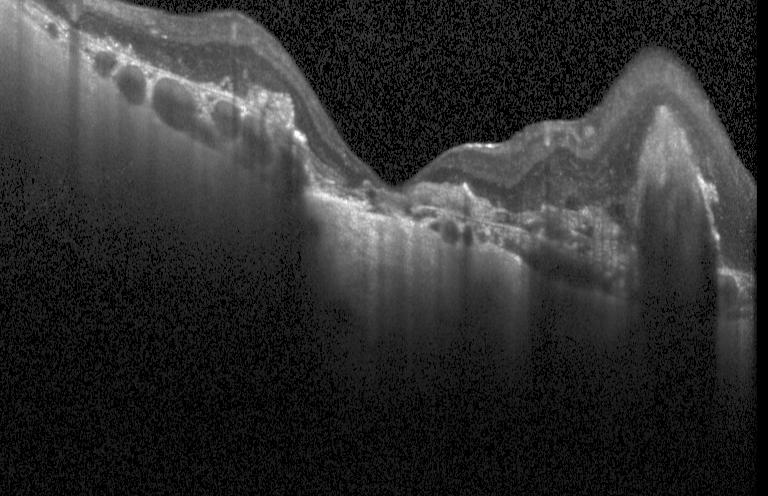
Instrument: Heidelberg Spectralis. Spectral-domain OCT. Optical coherence tomography scan. Horizontal scan through the fovea
The scan shows choroidal neovascularization (CNV).